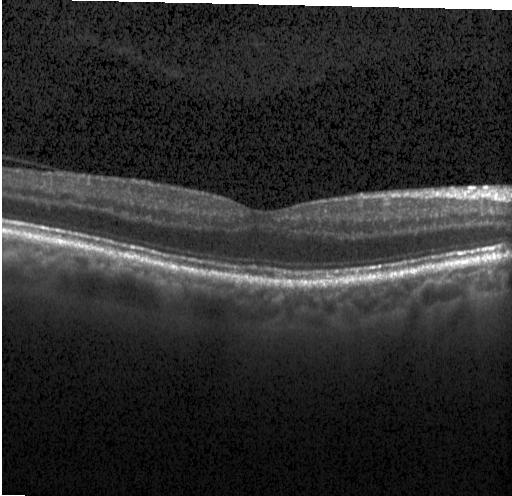

OCT finding: neither CNV, DME, nor drusen.